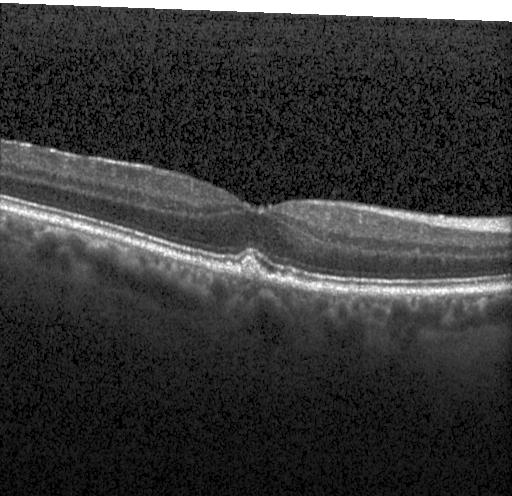 The scan shows multiple drusen.